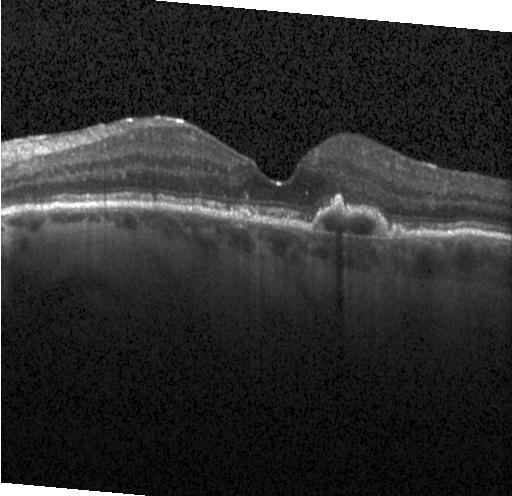
Heidelberg Spectralis, retinal OCT cross-section, spectral-domain OCT, through the macula.
Finding: choroidal neovascularization (CNV).